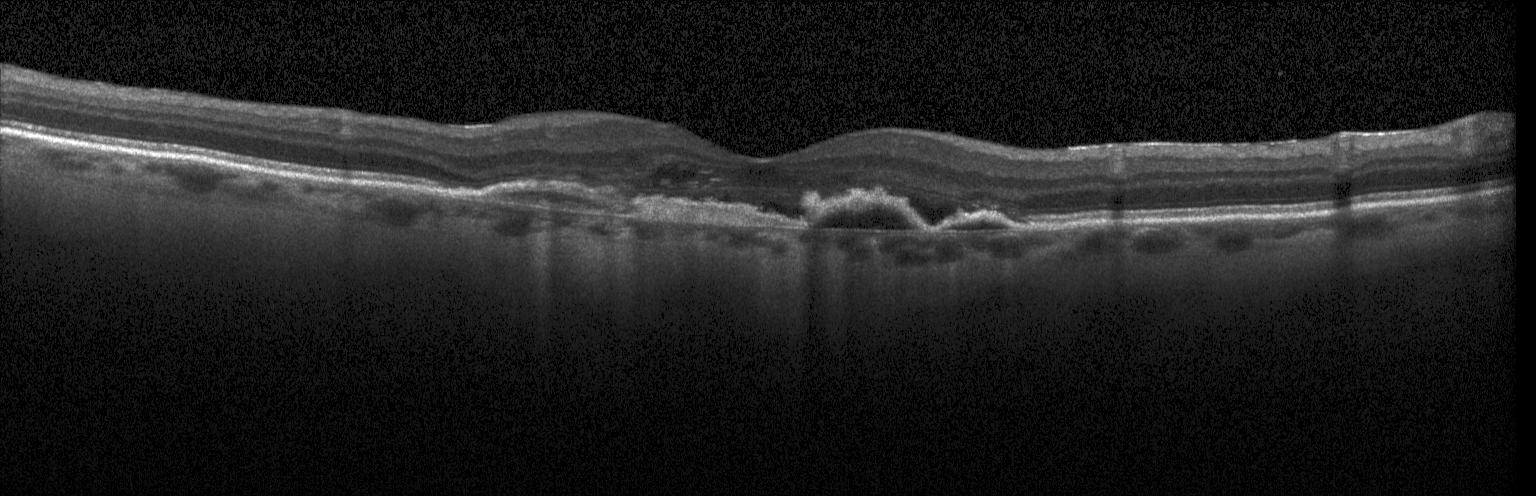
Diagnosis: a choroidal neovascular membrane.